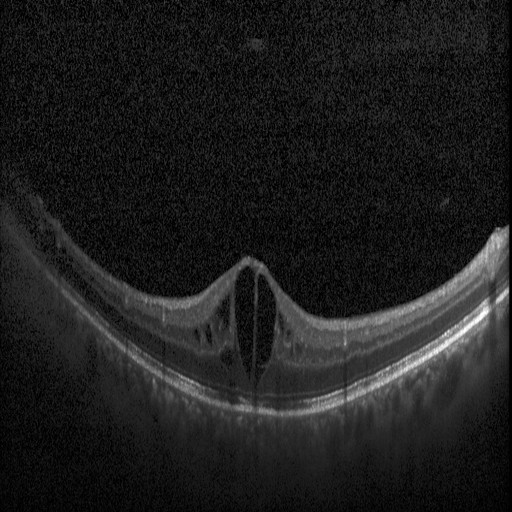

Retinal OCT B-scan — Impression: diabetic macular edema (DME).